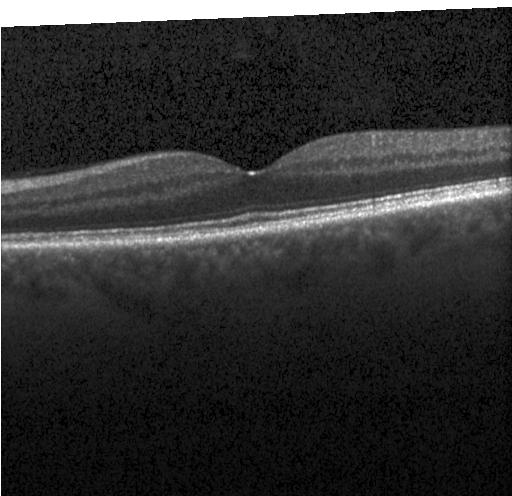

Heidelberg Spectralis OCT system · centered on the fovea · spectral-domain optical coherence tomography · optical coherence tomography B-scan. Impression: no CNV, no DME, and no drusen.